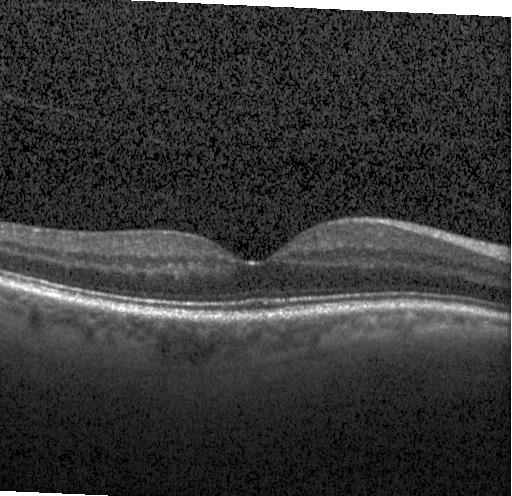 Retinal OCT B-scan, SD-OCT, instrument: Heidelberg Spectralis.
Finding: no CNV, DME, or drusen.